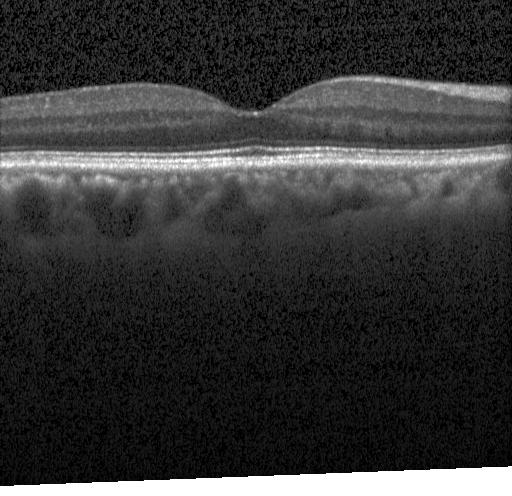
OCT finding: no CNV, no DME, and no drusen.